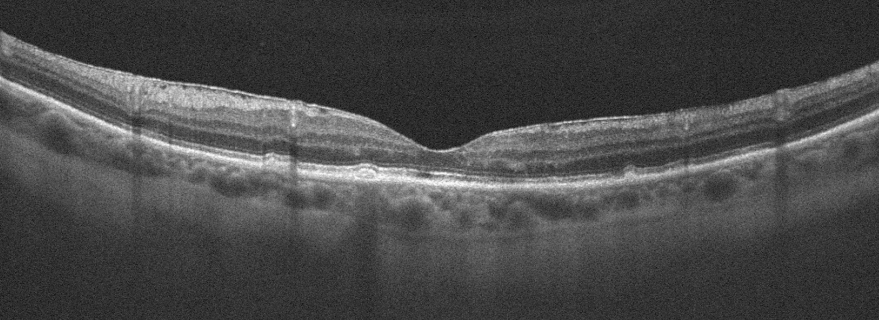 Macular scan; Optovue Avanti RTVue XR; optical coherence tomography scan. Macular OCT: ERM.